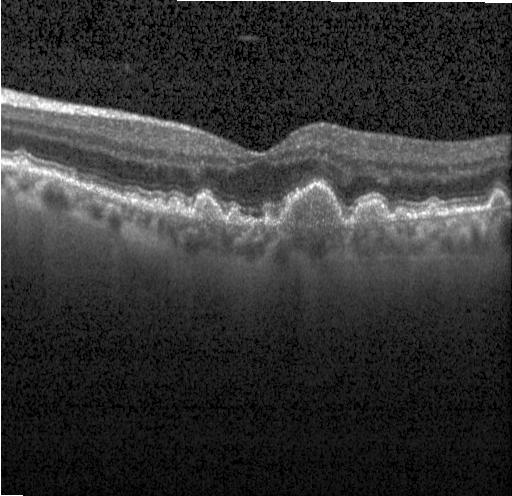

Macular scan. Instrument: Heidelberg Spectralis. Optical coherence tomography scan — Multiple drusen.